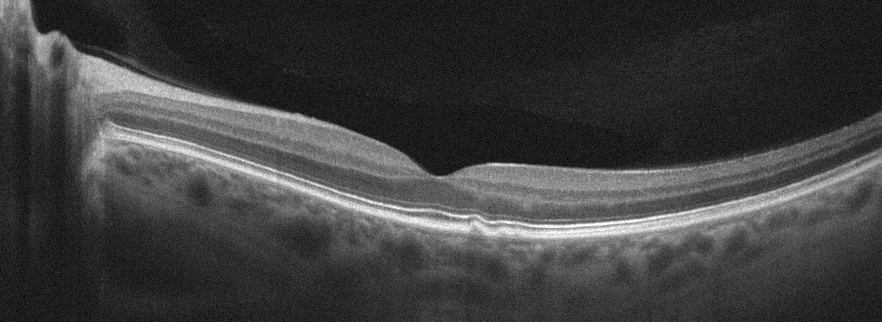
Left eye. OCT line scan
Macular OCT: age-related macular degeneration.